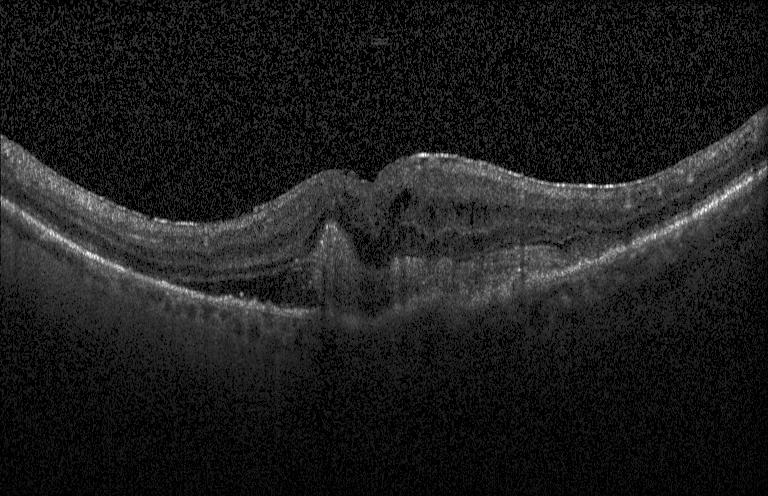 Assessment: choroidal neovascularization.